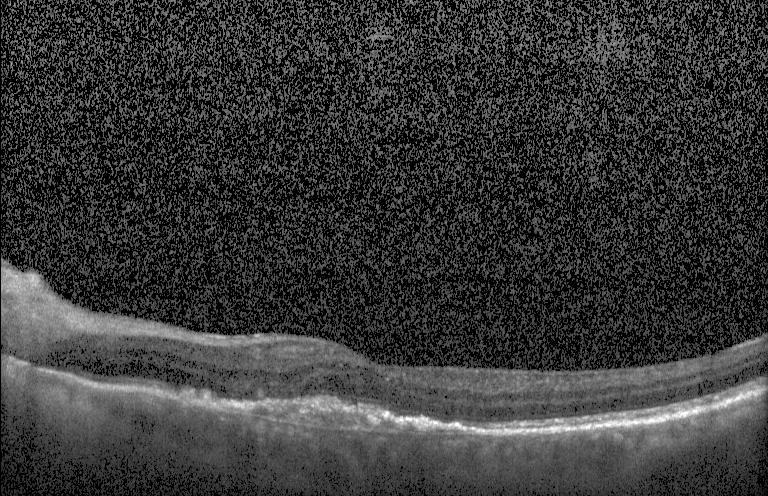 OCT B-scan — OCT finding: choroidal neovascularization.